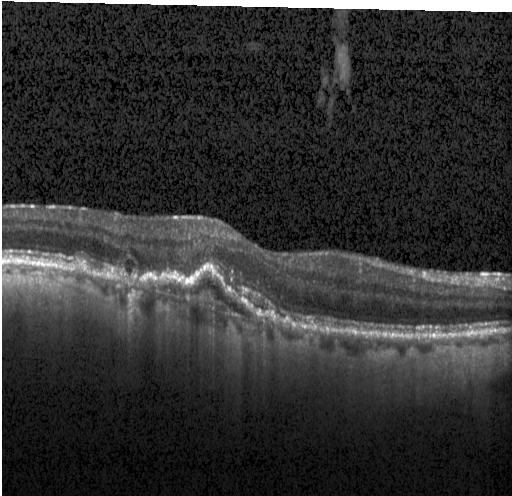

OCT line scan · horizontal scan through the fovea
Impression: a choroidal neovascular membrane.